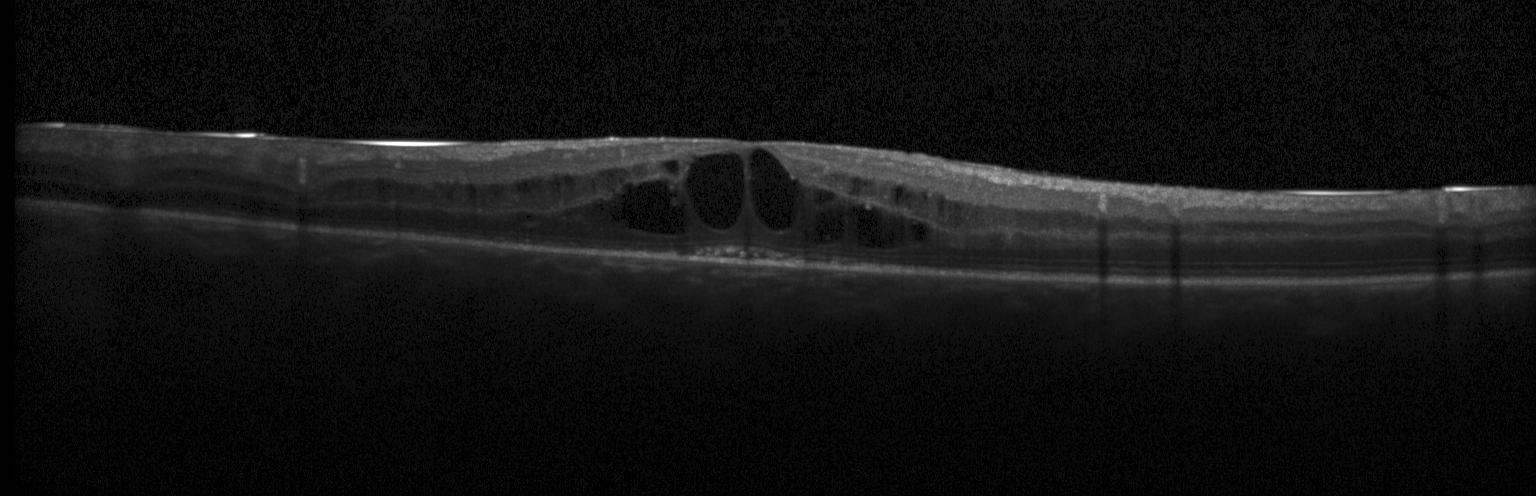

Diagnosis: DME.